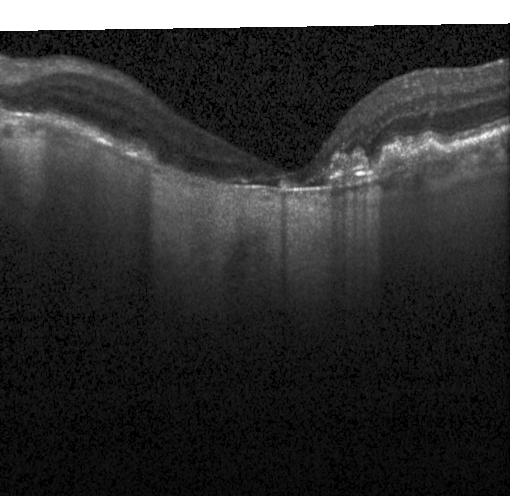
Retinal OCT B-scan.
This B-scan demonstrates choroidal neovascularization (CNV).